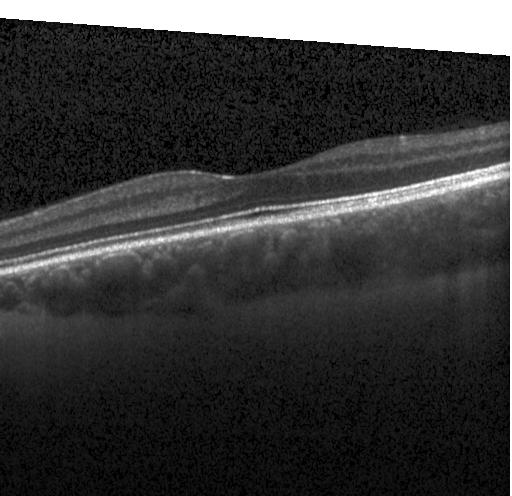

Spectral-domain OCT · horizontal scan through the fovea · retinal OCT cross-section · Heidelberg Spectralis OCT system.
Diagnosis: neither choroidal neovascularization, diabetic macular edema, nor drusen.